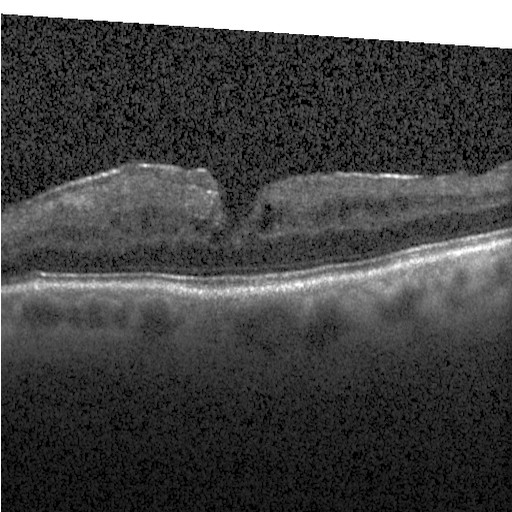
OCT scan showing DME.